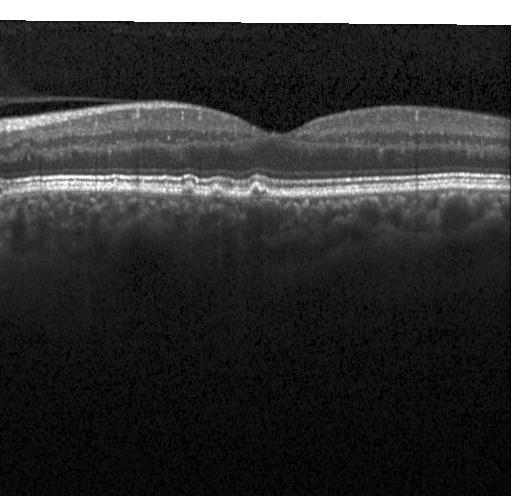

Optical coherence tomography scan; through the macula — Assessment: multiple drusen.